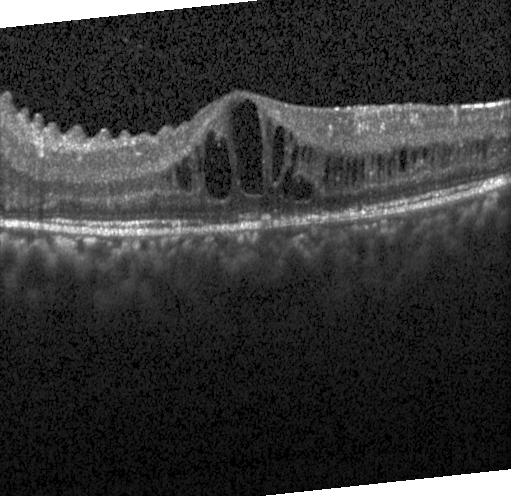 This B-scan demonstrates DME.